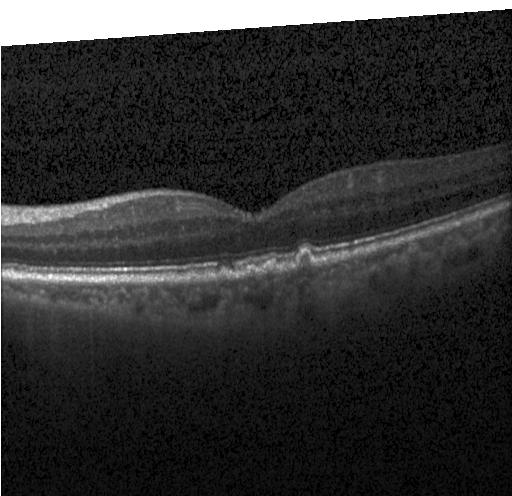
OCT line scan · macular scan — Sub-RPE drusenoid deposits.